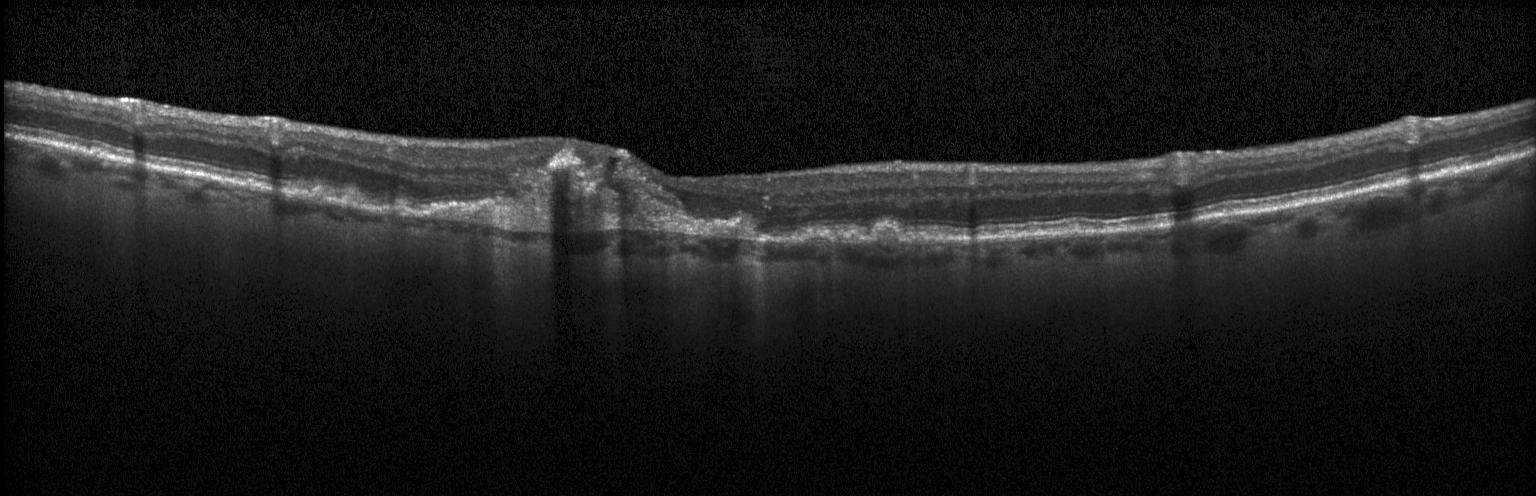 Heidelberg Spectralis. Spectral-domain OCT. Fovea-centered. OCT B-scan — Finding: a choroidal neovascular membrane.